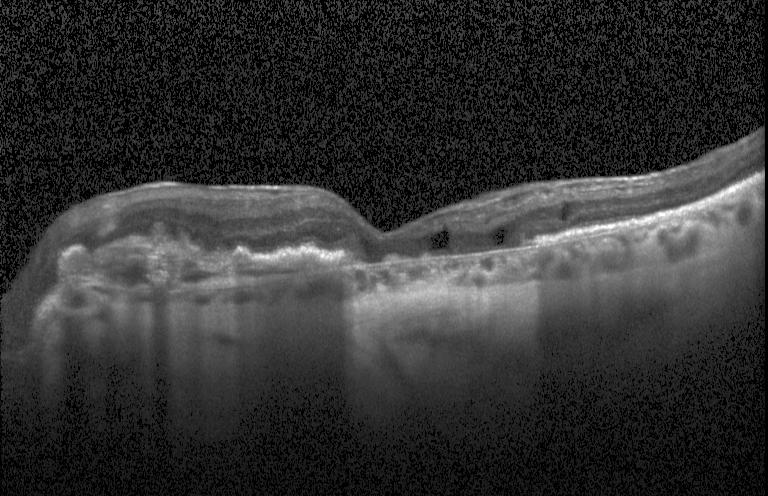

Macular scan. Optical coherence tomography B-scan. Assessment: choroidal neovascularization.